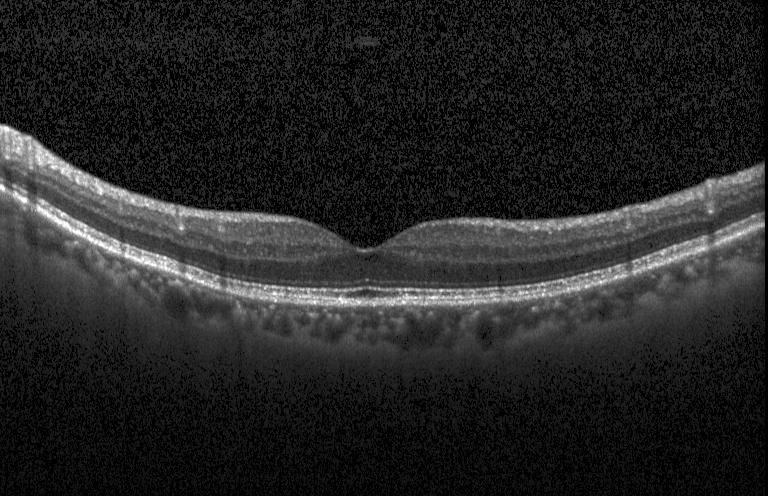 Retinal OCT cross-section showing no evidence of choroidal neovascularization, diabetic macular edema, or drusen.